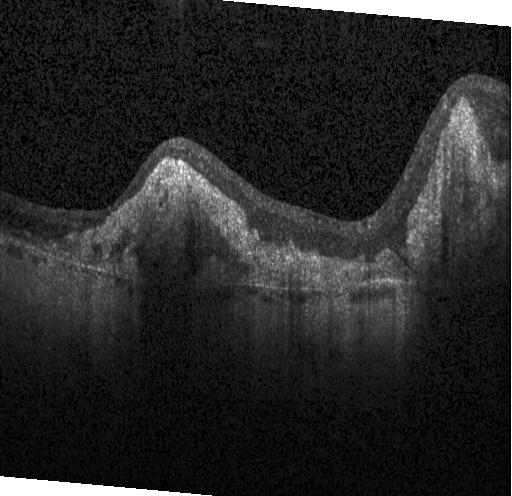 Spectral-domain OCT B-scan: a choroidal neovascular membrane.